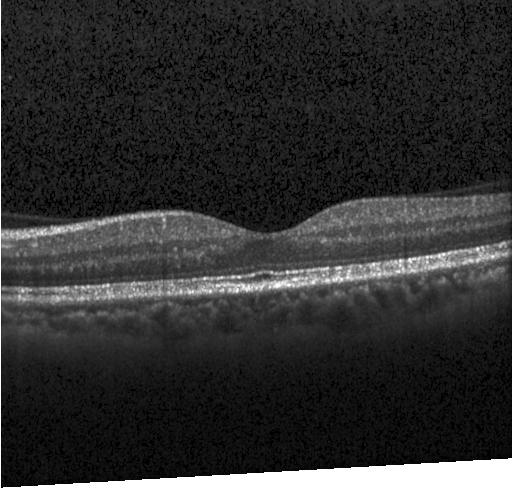
Through the macula; OCT B-scan — OCT finding: no choroidal neovascularization, diabetic macular edema, or drusen.